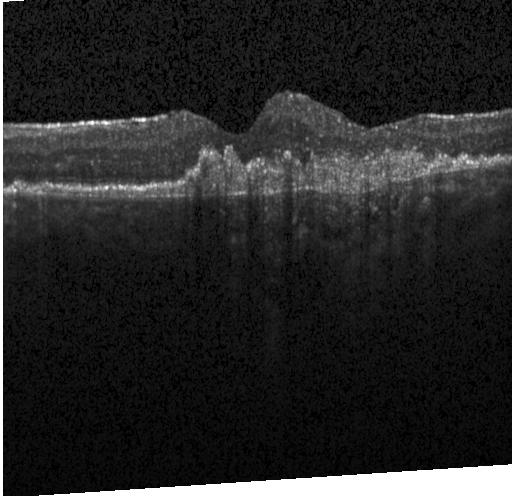

Impression: a choroidal neovascular membrane.